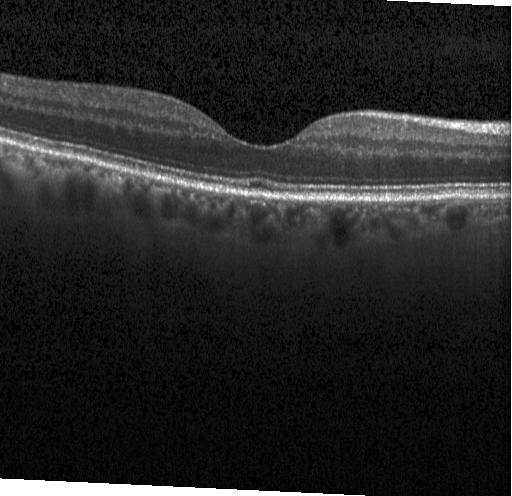
Centered on the fovea; retinal OCT cross-section; Heidelberg Spectralis; spectral-domain OCT.
Finding: no CNV, DME, or drusen.